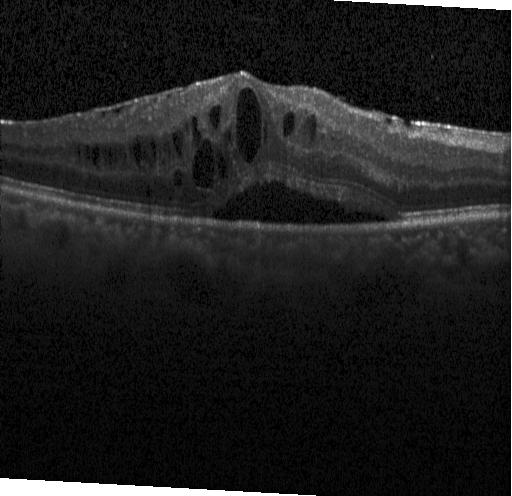

Impression: diabetic macular edema (DME).